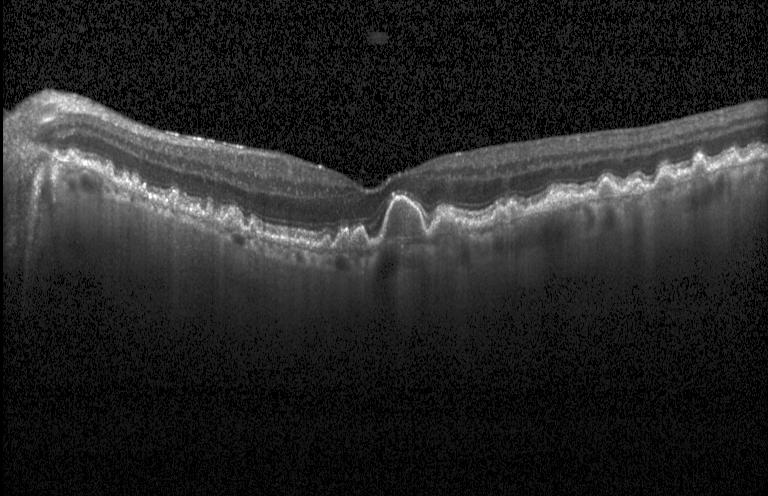
Diagnosis: multiple drusen.